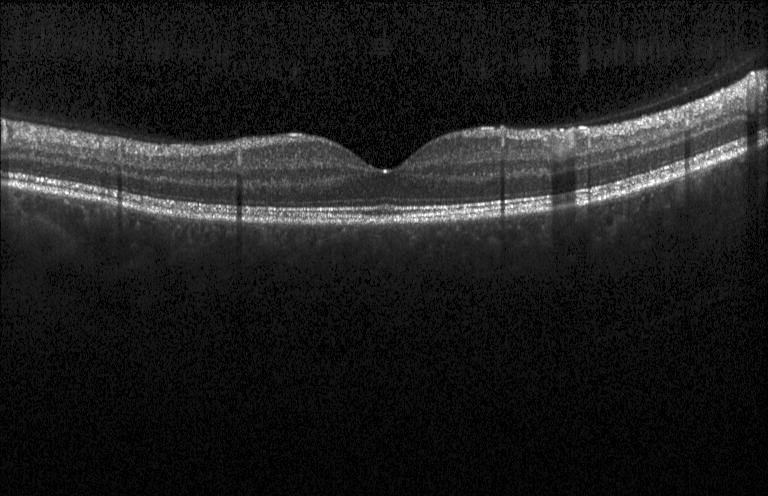 OCT line scan — Impression: neither choroidal neovascularization, diabetic macular edema, nor drusen.